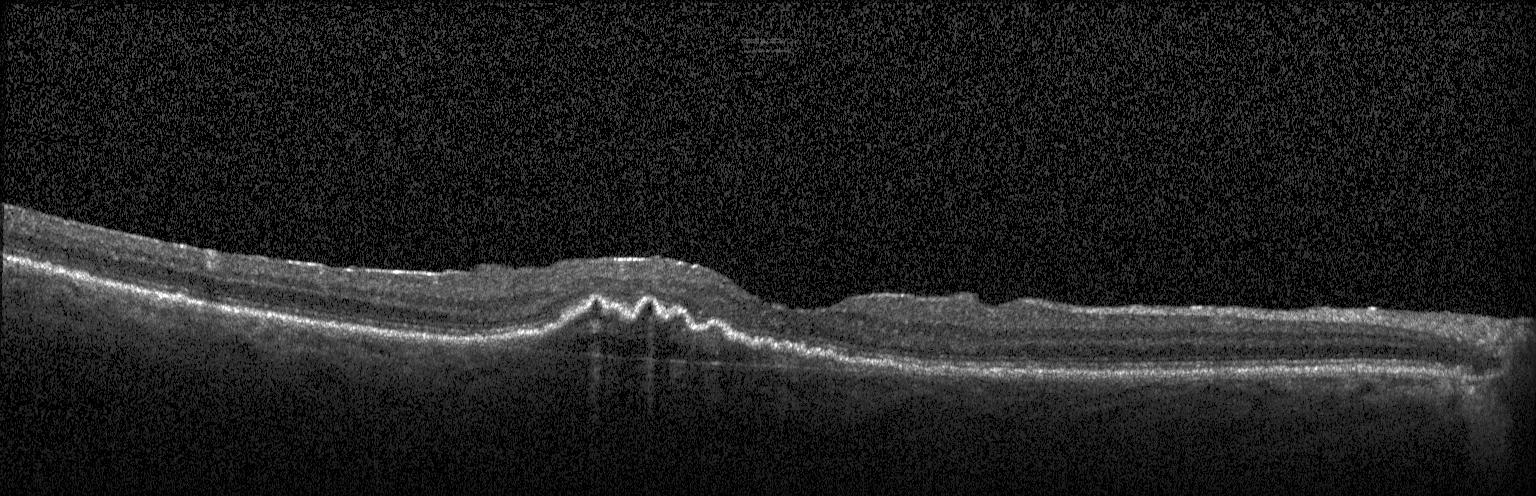 Heidelberg Spectralis OCT system · optical coherence tomography scan · fovea-centered.
OCT finding: a choroidal neovascular membrane.